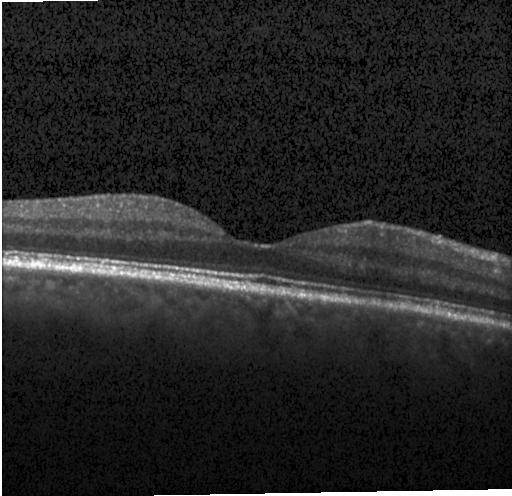
Centered on the fovea. Heidelberg Spectralis OCT system. Retinal OCT cross-section. SD-OCT.
OCT finding: no choroidal neovascularization, diabetic macular edema, or drusen.